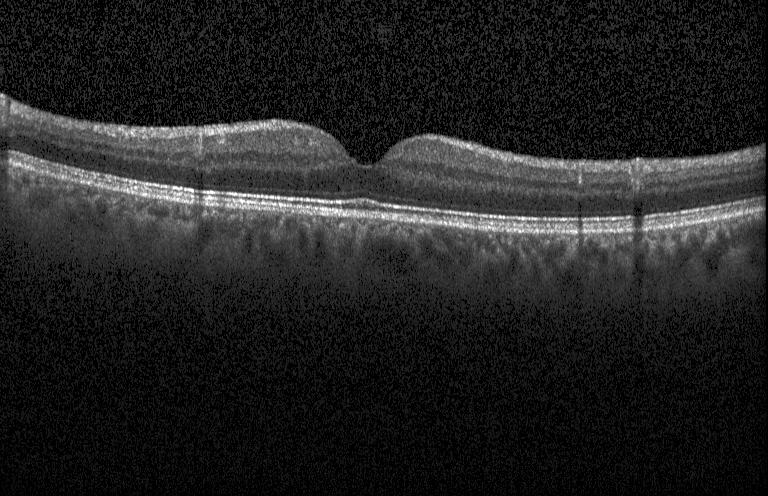
Diagnosis: no choroidal neovascularization, diabetic macular edema, or drusen.